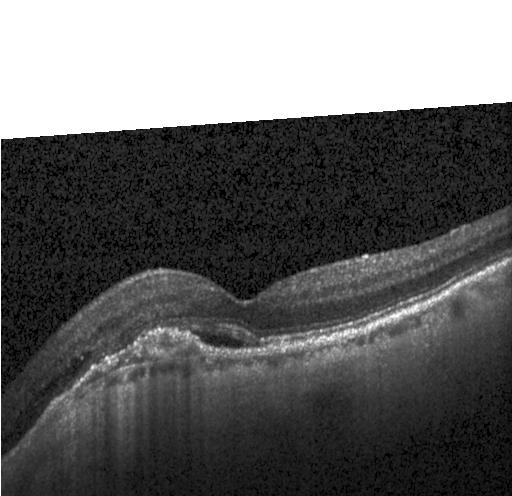

OCT B-scan — Diagnosis: a choroidal neovascular membrane.